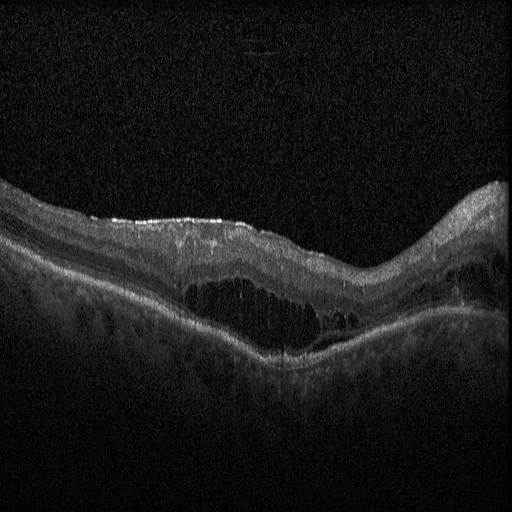 OCT line scan.
The scan shows diabetic macular edema.